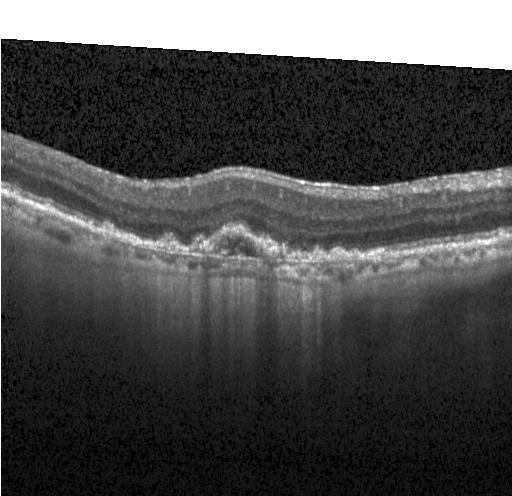

Retinal OCT cross-section showing choroidal neovascularization (CNV).